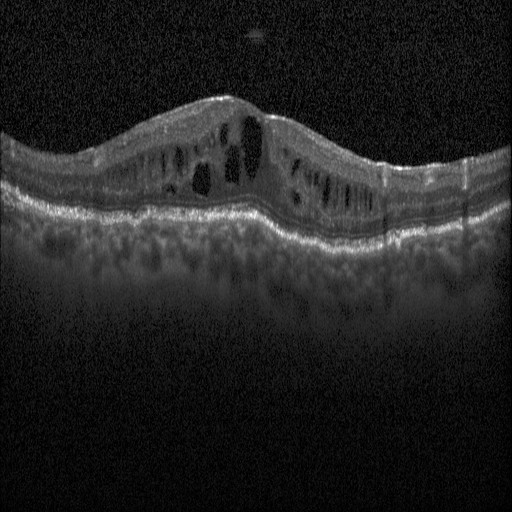 Diagnosis: diabetic macular edema (DME).